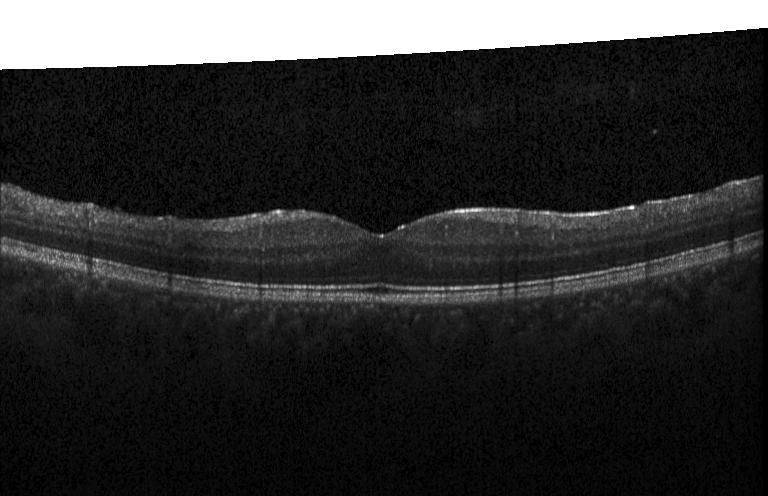 OCT B-scan · instrument: Heidelberg Spectralis · SD-OCT · through the macula.
Impression: neither CNV, DME, nor drusen.